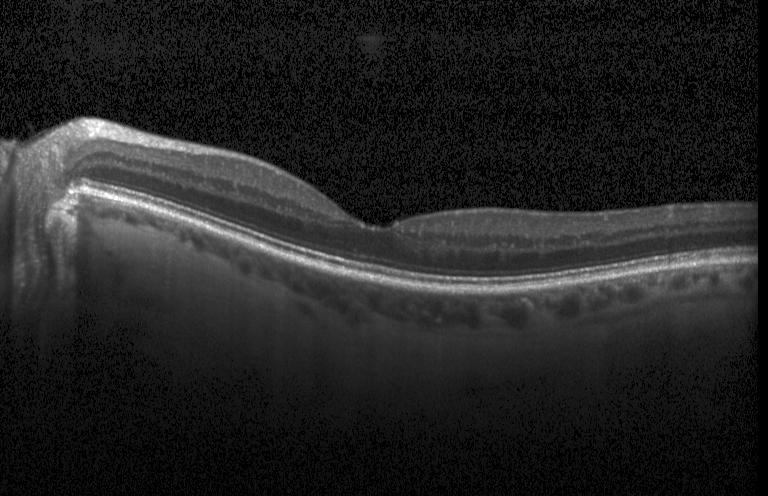 Spectral-domain OCT B-scan: neither CNV, DME, nor drusen.